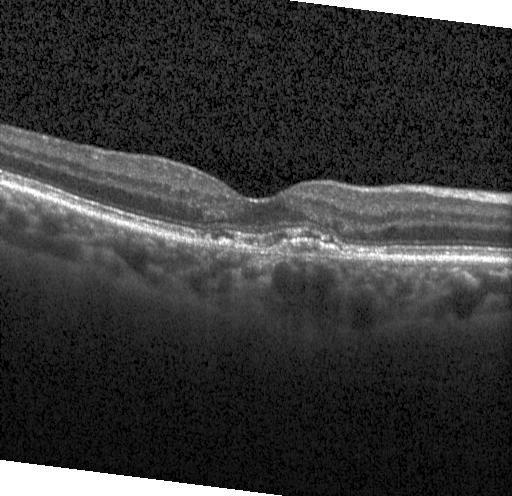 OCT B-scan
The scan shows a choroidal neovascular membrane.